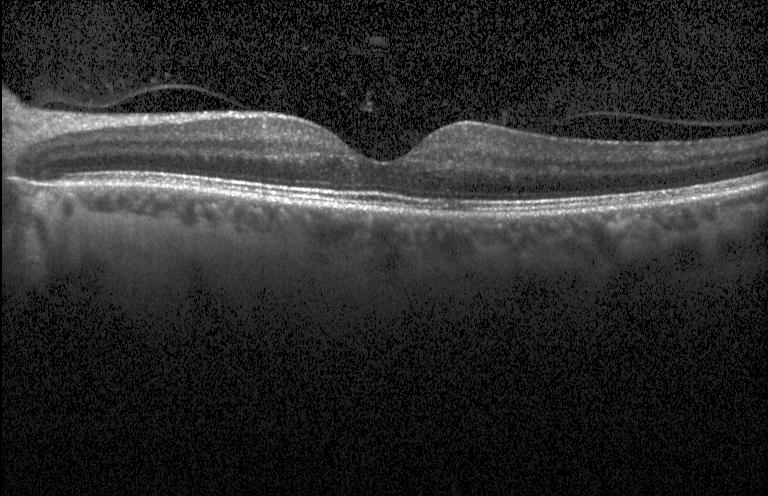 Retinal OCT B-scan. Heidelberg Spectralis
This B-scan demonstrates no choroidal neovascularization, diabetic macular edema, or drusen.